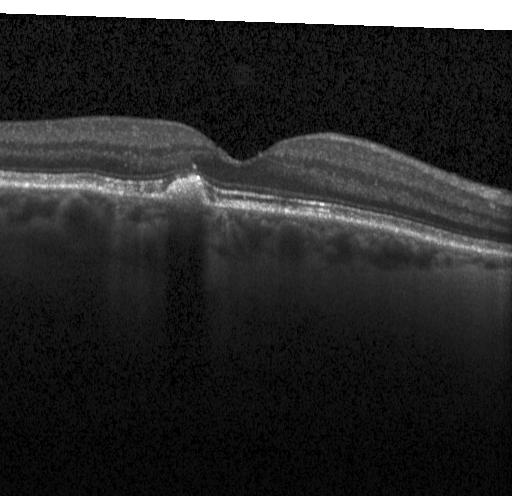 OCT finding: sub-RPE drusenoid deposits.